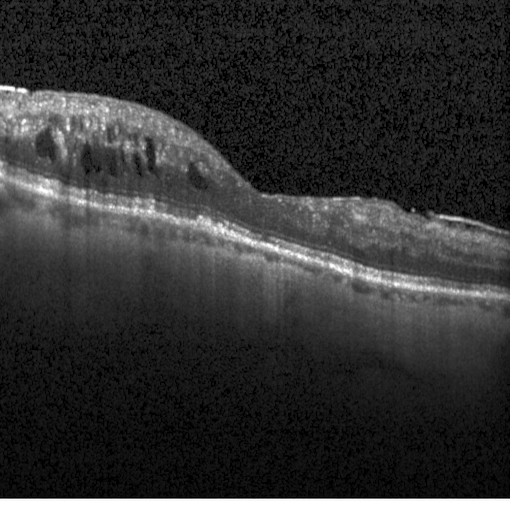 Macular OCT demonstrating DME.